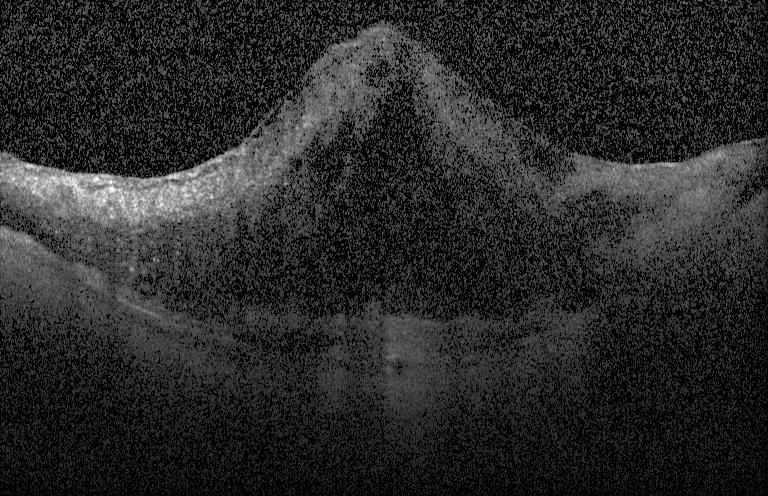

Retinal OCT B-scan.
Assessment: choroidal neovascularization (CNV).